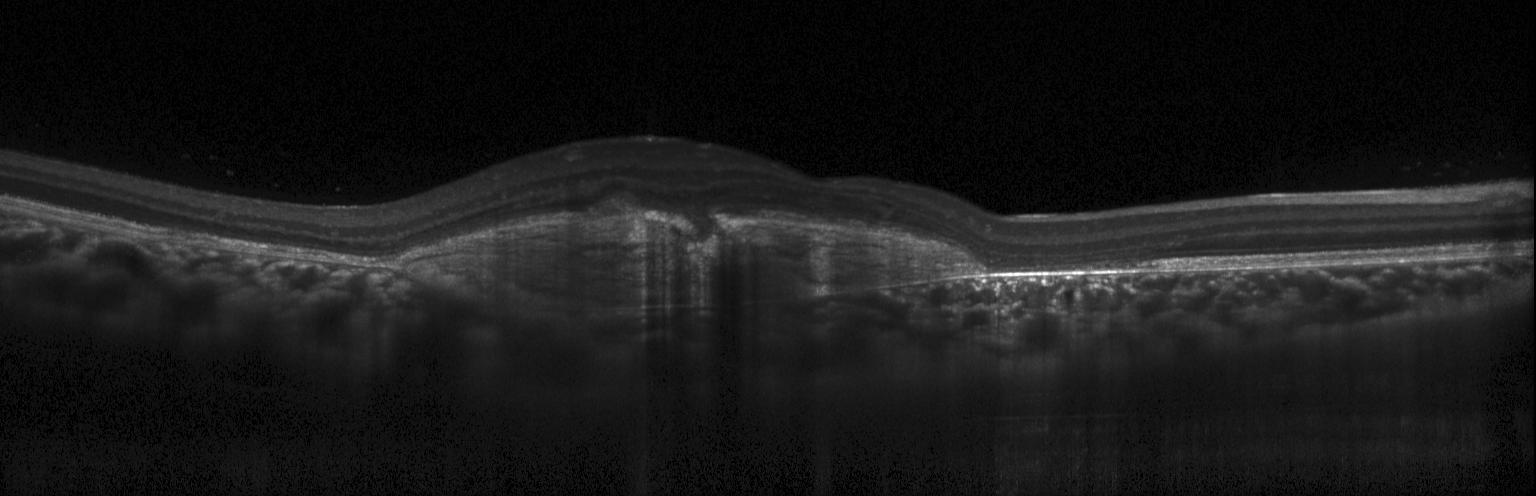

Heidelberg Spectralis. Optical coherence tomography scan. SD-OCT. A choroidal neovascular membrane.